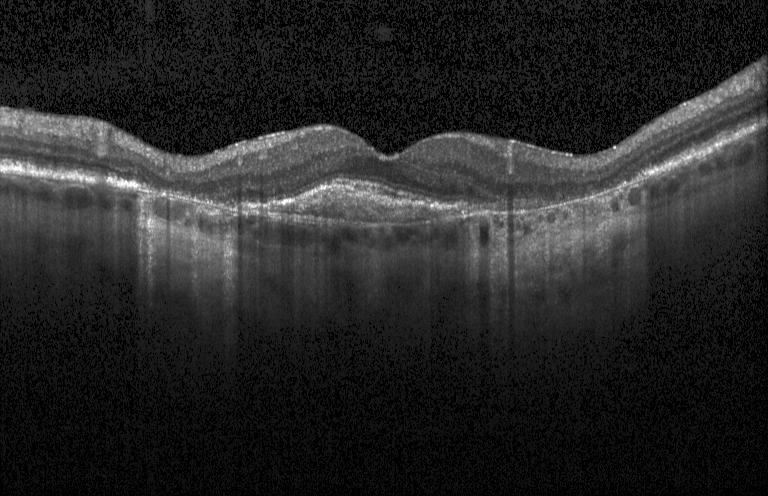

OCT line scan. Finding: choroidal neovascularization.